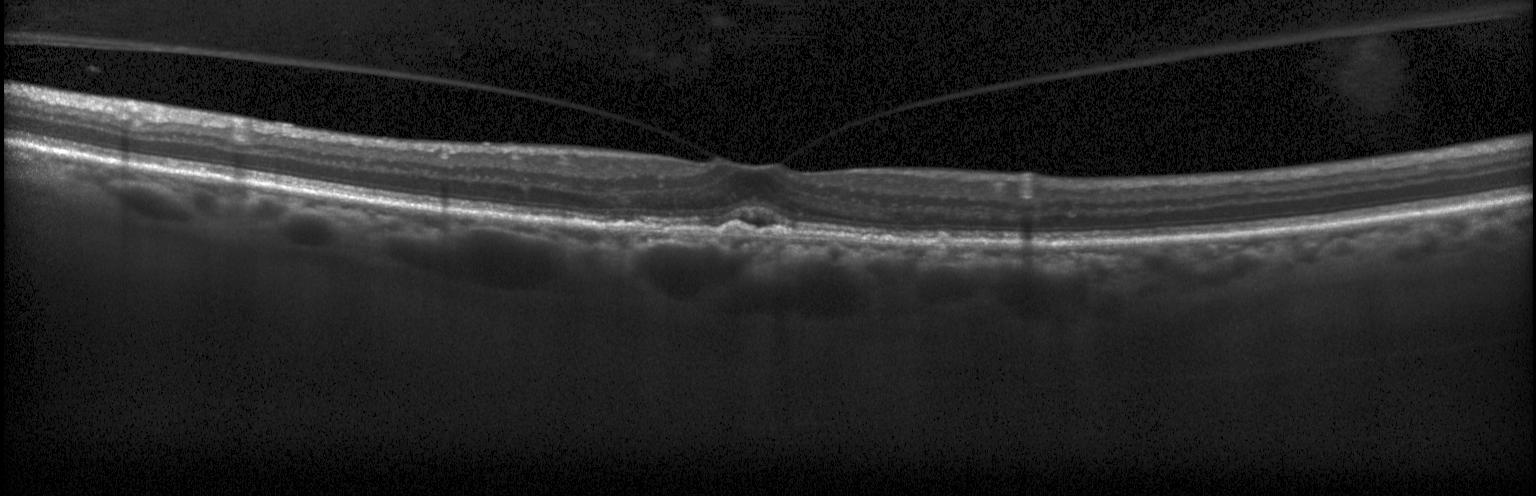 Heidelberg Spectralis, retinal OCT B-scan — The scan shows a choroidal neovascular membrane.